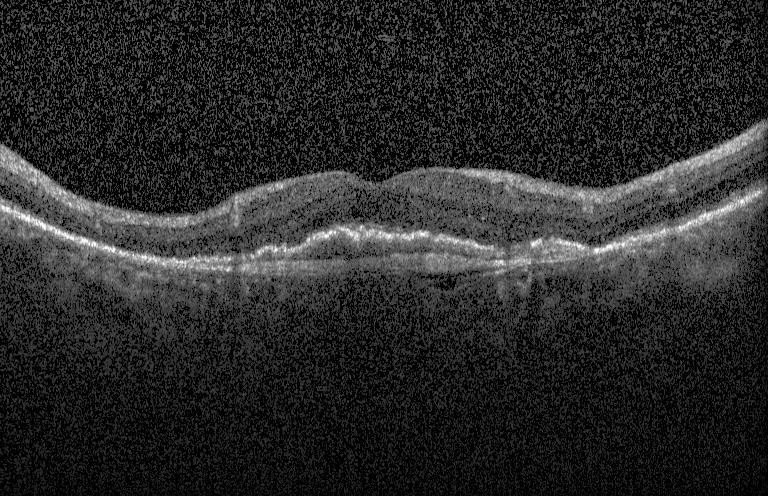 Finding: choroidal neovascularization.